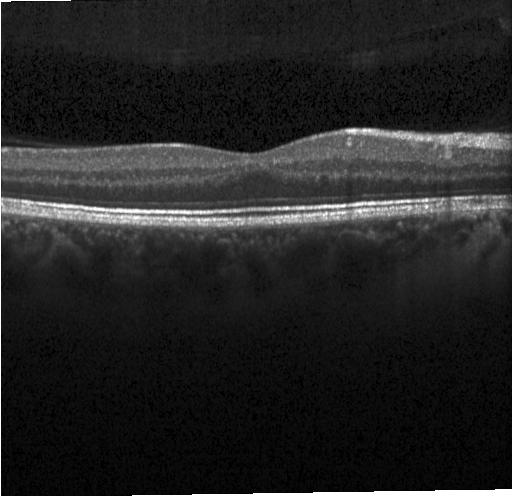

Retinal OCT cross-section showing neither choroidal neovascularization, diabetic macular edema, nor drusen.